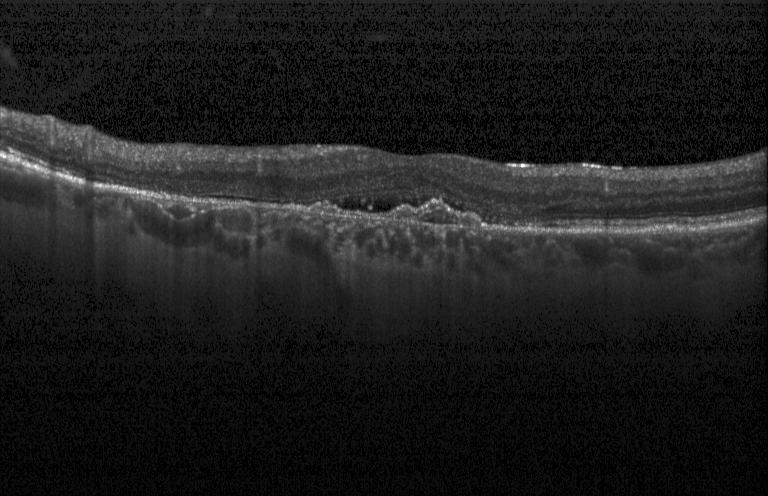
OCT B-scan.
A choroidal neovascular membrane.